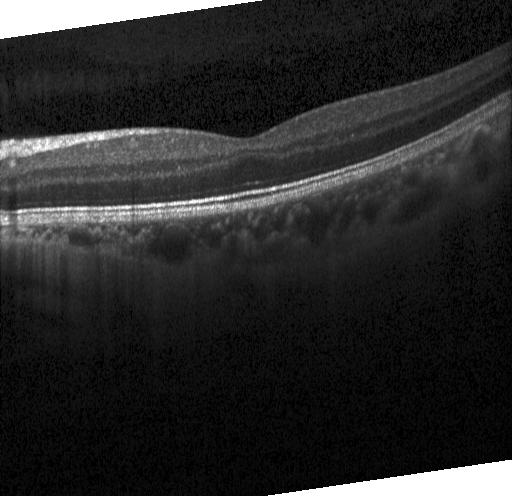

SD-OCT, Heidelberg Spectralis OCT system, macular scan, retinal OCT cross-section.
Assessment: no choroidal neovascularization, no diabetic macular edema, and no drusen.